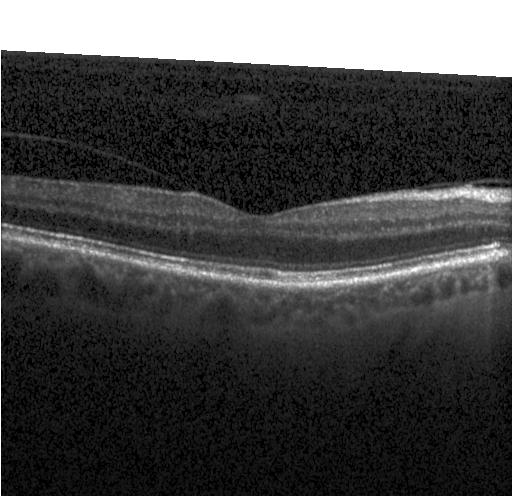

Retinal OCT B-scan, fovea-centered, SD-OCT.
Impression: no evidence of choroidal neovascularization, diabetic macular edema, or drusen.